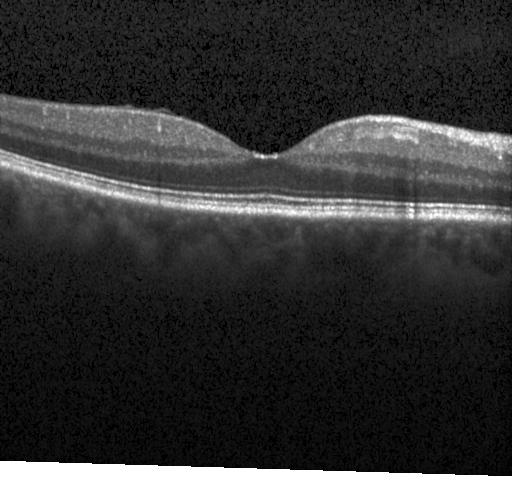 Impression: no choroidal neovascularization, diabetic macular edema, or drusen.